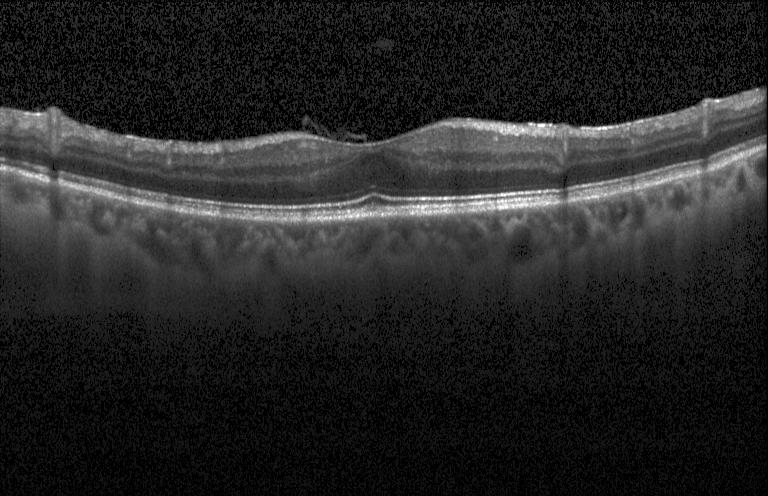 Macular OCT: no CNV, DME, or drusen.